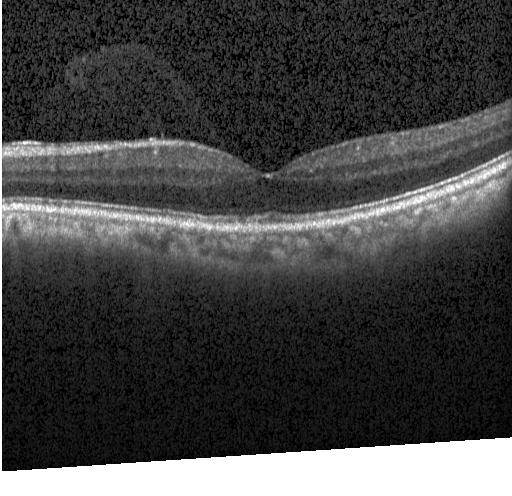 Optical coherence tomography scan. Finding: no CNV, no DME, and no drusen.